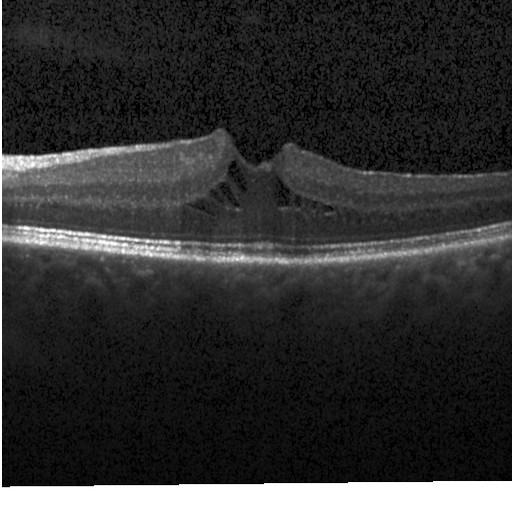 Optical coherence tomography B-scan, acquired on a Heidelberg Spectralis, spectral-domain OCT.
Impression: diabetic macular edema.